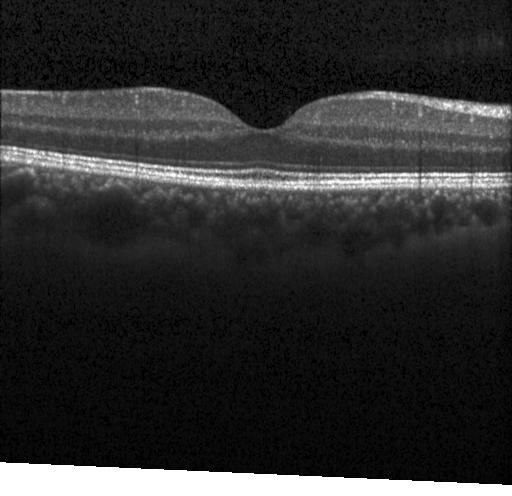
Spectral-domain optical coherence tomography · centered on the fovea · acquired on a Heidelberg Spectralis · retinal OCT B-scan.
Diagnosis: neither CNV, DME, nor drusen.